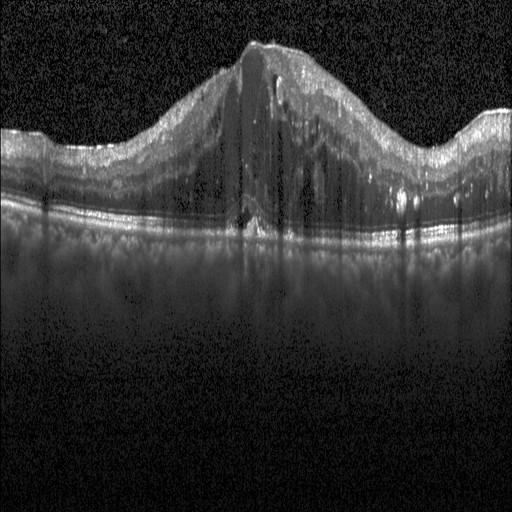 Assessment: diabetic macular edema.